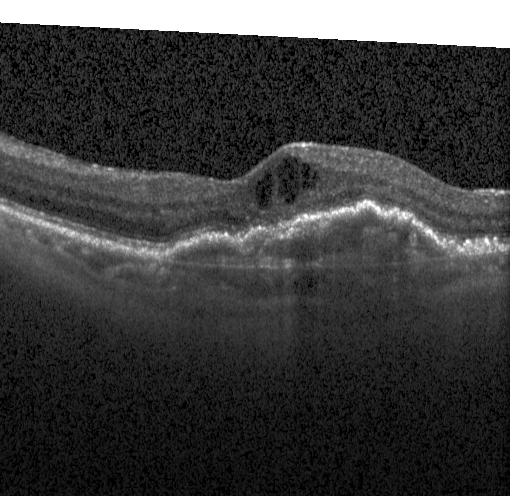 A choroidal neovascular membrane.